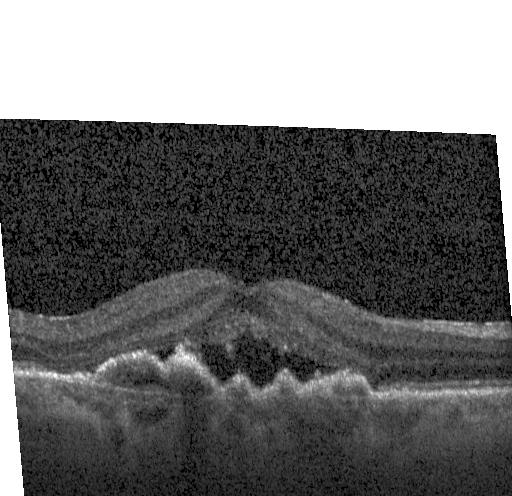

Acquired on a Heidelberg Spectralis · spectral-domain optical coherence tomography · optical coherence tomography scan · through the macula
Impression: a choroidal neovascular membrane.